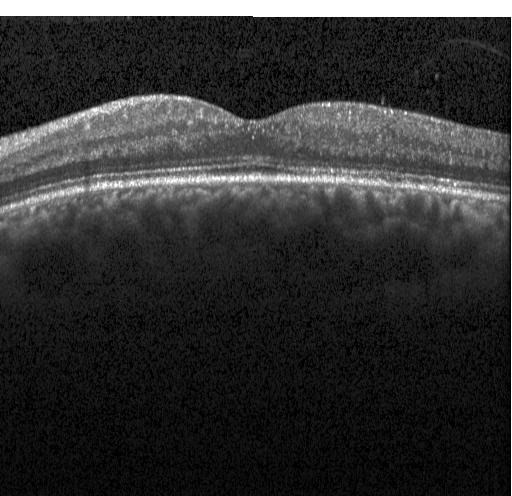

Spectral-domain optical coherence tomography; retinal OCT cross-section.
Dx: neither choroidal neovascularization, diabetic macular edema, nor drusen.